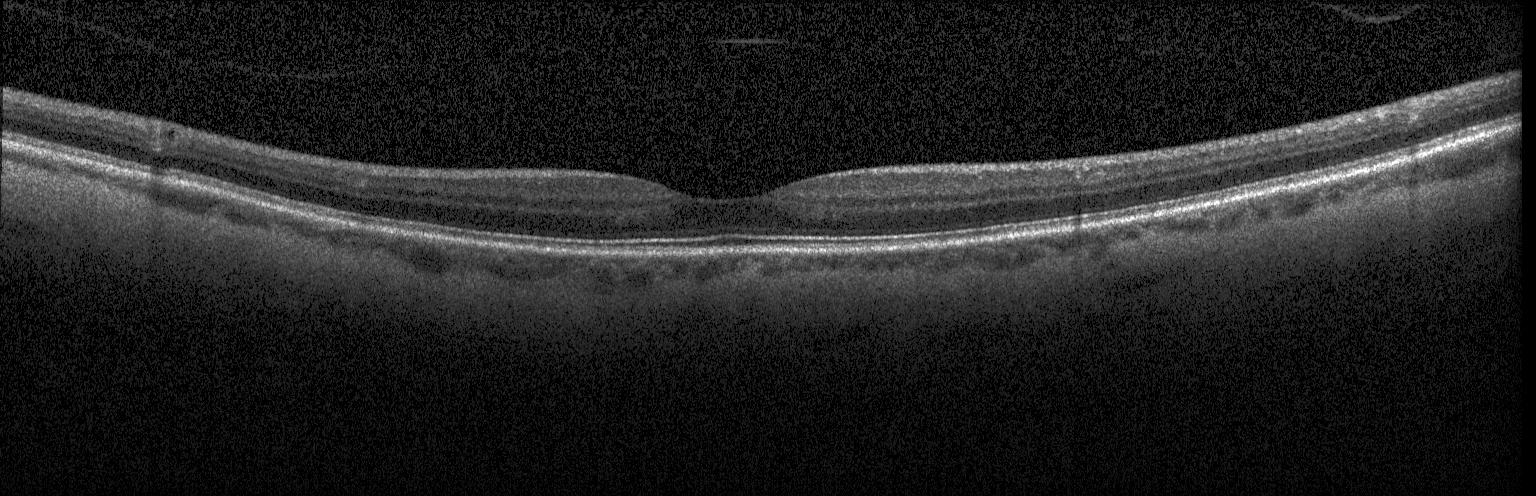 Optical coherence tomography scan; macular scan; Heidelberg Spectralis; SD-OCT
This B-scan demonstrates neither choroidal neovascularization, diabetic macular edema, nor drusen.